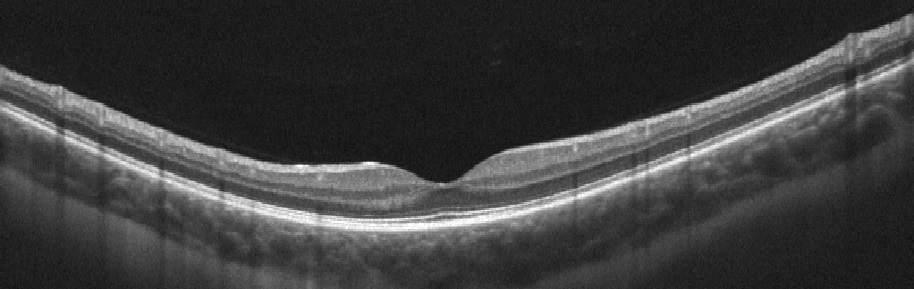
Dx: no evidence of AMD, DME, ERM, RAO, RVO, or VID.